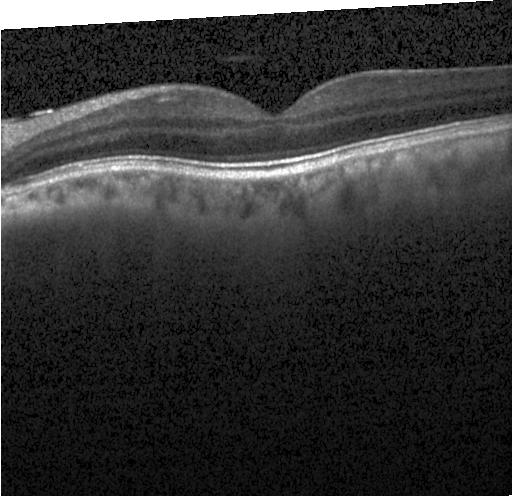 Spectral-domain optical coherence tomography. Optical coherence tomography B-scan. Through the macula.
Assessment: neither CNV, DME, nor drusen.